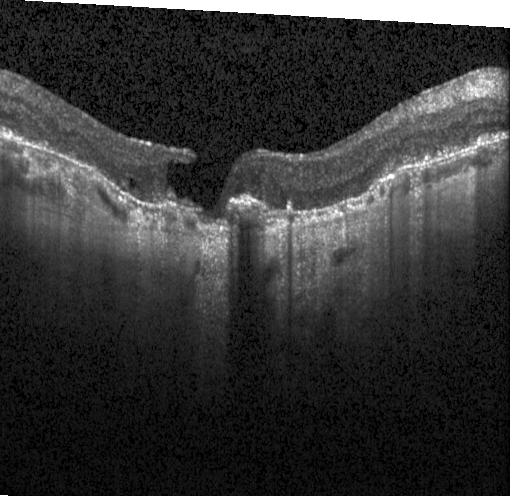

Heidelberg Spectralis, optical coherence tomography scan, SD-OCT
Assessment: CNV.